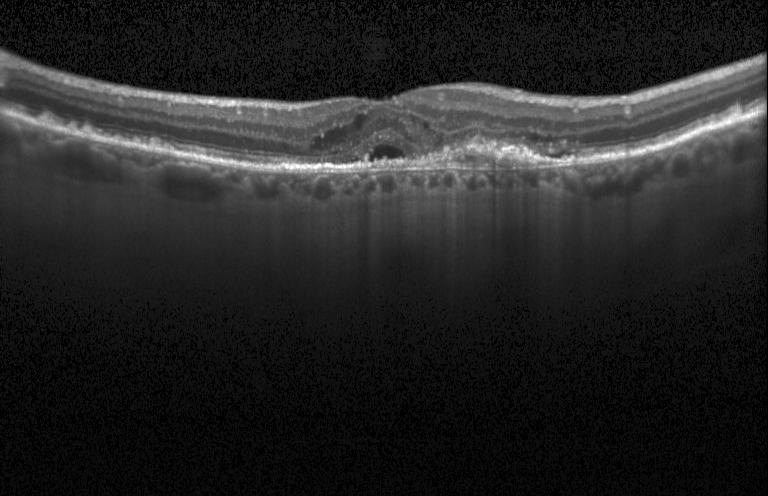
Retinal OCT cross-section showing choroidal neovascularization (CNV).